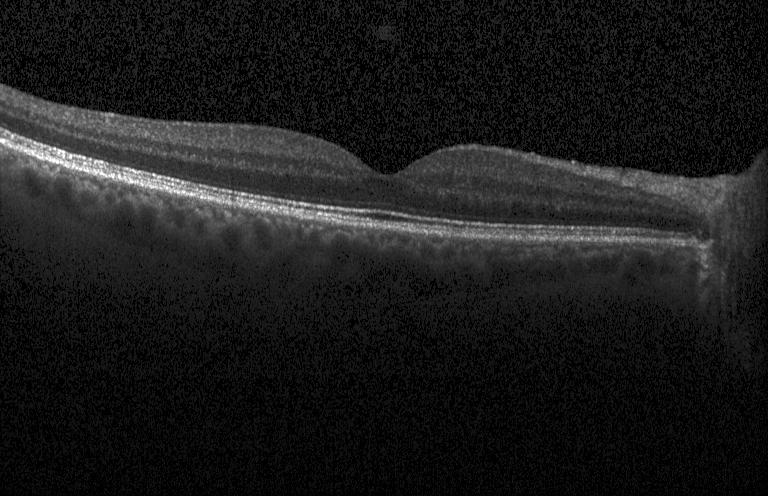
Retinal OCT cross-section · Heidelberg Spectralis OCT system.
No choroidal neovascularization, no diabetic macular edema, and no drusen.